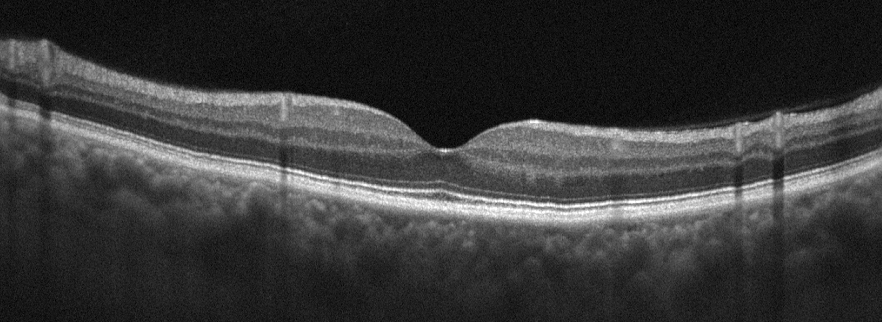
Optovue Avanti RTVue XR; right eye; OCT line scan.
Diagnosis: absence of AMD, DME, ERM, RAO, RVO, and vitreomacular interface disease.